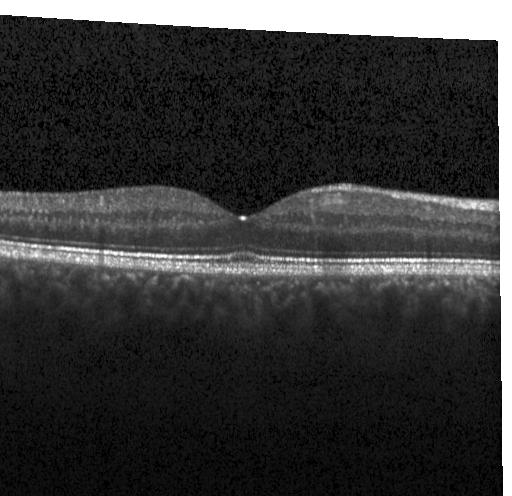
Finding: no evidence of choroidal neovascularization, diabetic macular edema, or drusen.